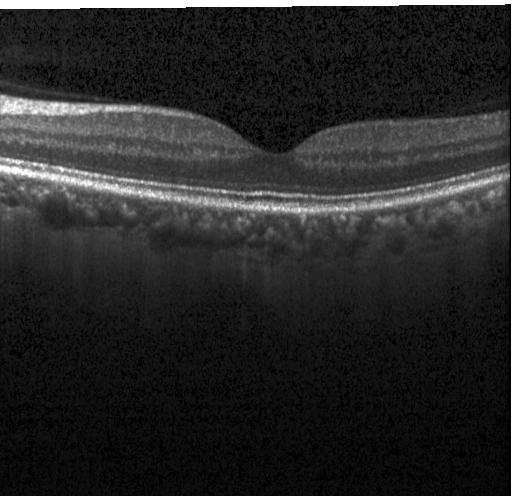
Retinal OCT cross-section — This B-scan demonstrates no choroidal neovascularization, no diabetic macular edema, and no drusen.